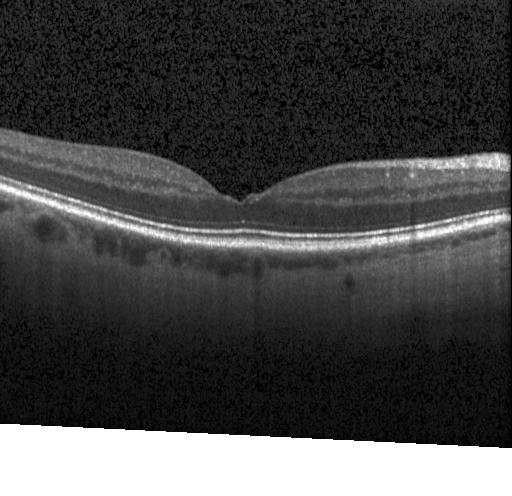
OCT B-scan. No choroidal neovascularization, no diabetic macular edema, and no drusen.